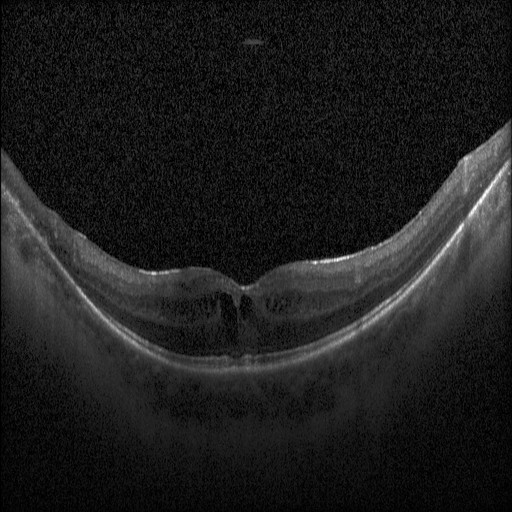
Heidelberg Spectralis · optical coherence tomography B-scan — The scan shows diabetic macular edema (DME).